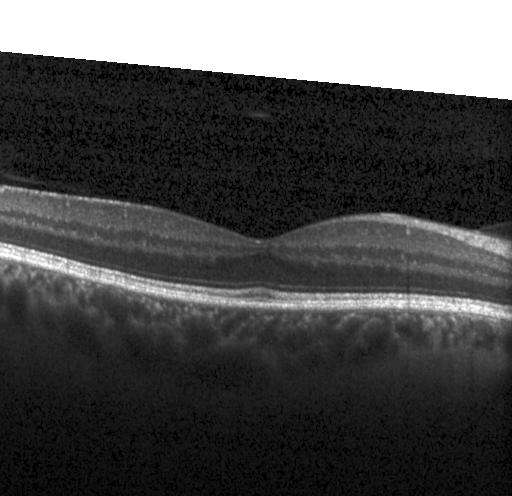

Macular OCT: neither choroidal neovascularization, diabetic macular edema, nor drusen.